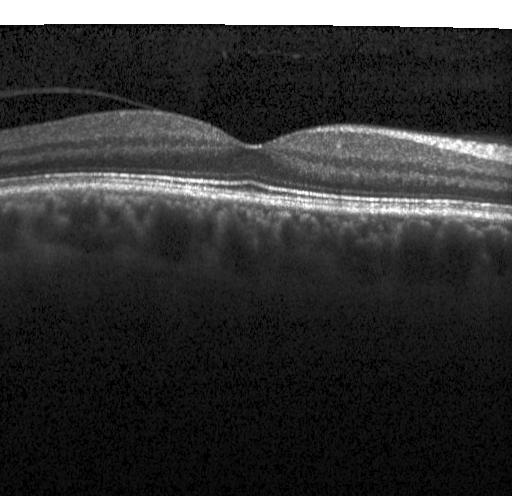

OCT B-scan · instrument: Heidelberg Spectralis.
Macular OCT: no choroidal neovascularization, diabetic macular edema, or drusen.